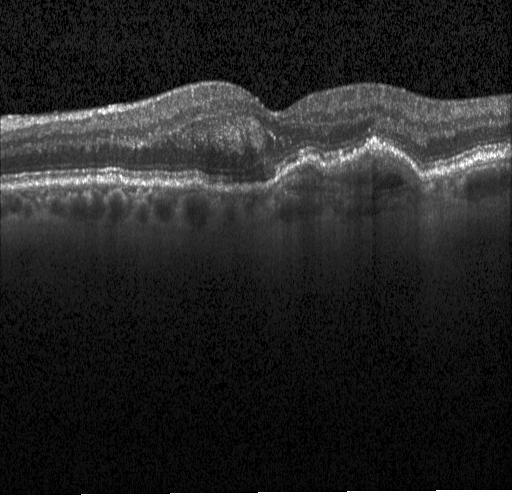
Dx: CNV.